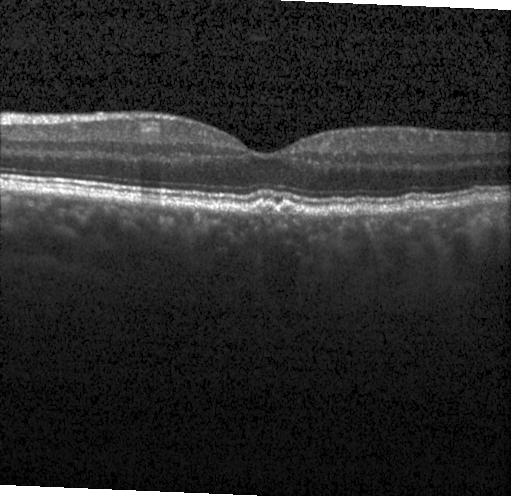
Spectral-domain optical coherence tomography, instrument: Heidelberg Spectralis, centered on the fovea, retinal OCT B-scan. The scan shows drusen.